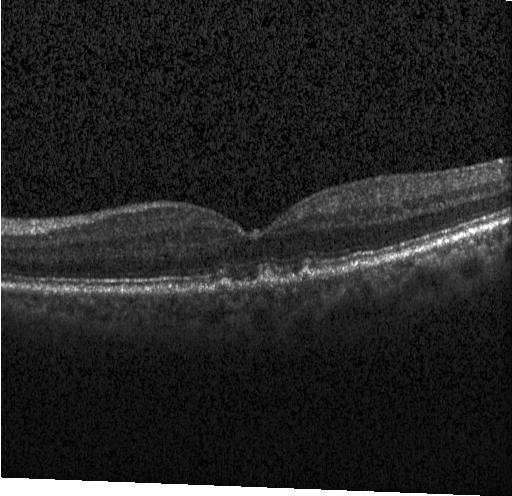

OCT scan showing sub-RPE drusenoid deposits.